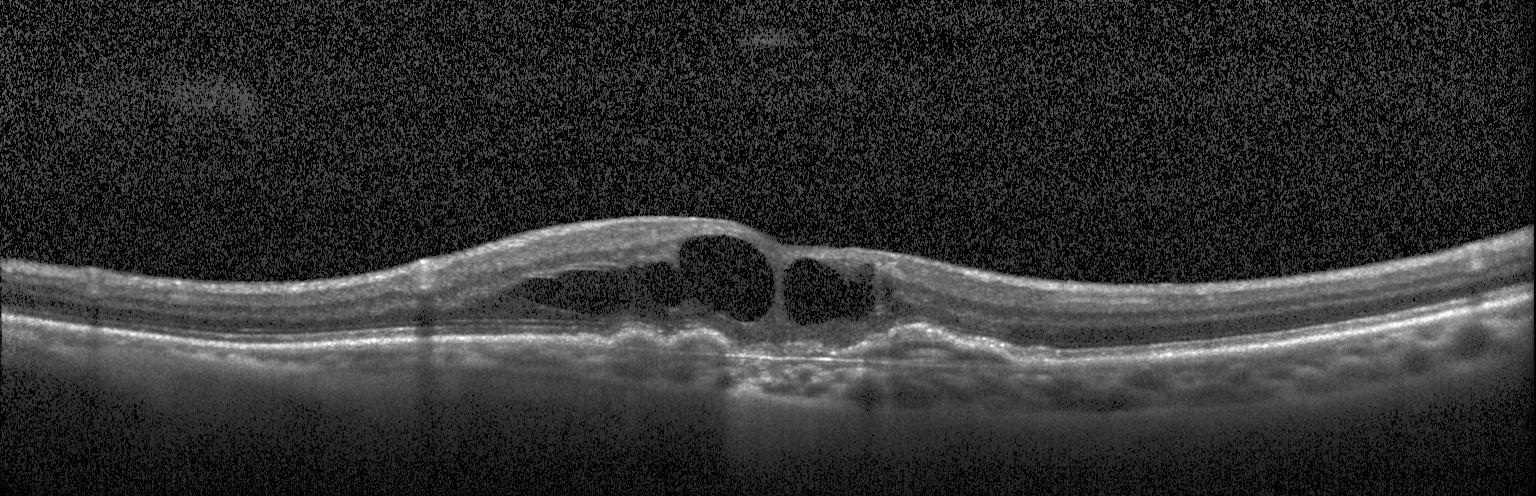

Optical coherence tomography scan. Acquired on a Heidelberg Spectralis. Finding: choroidal neovascularization (CNV).